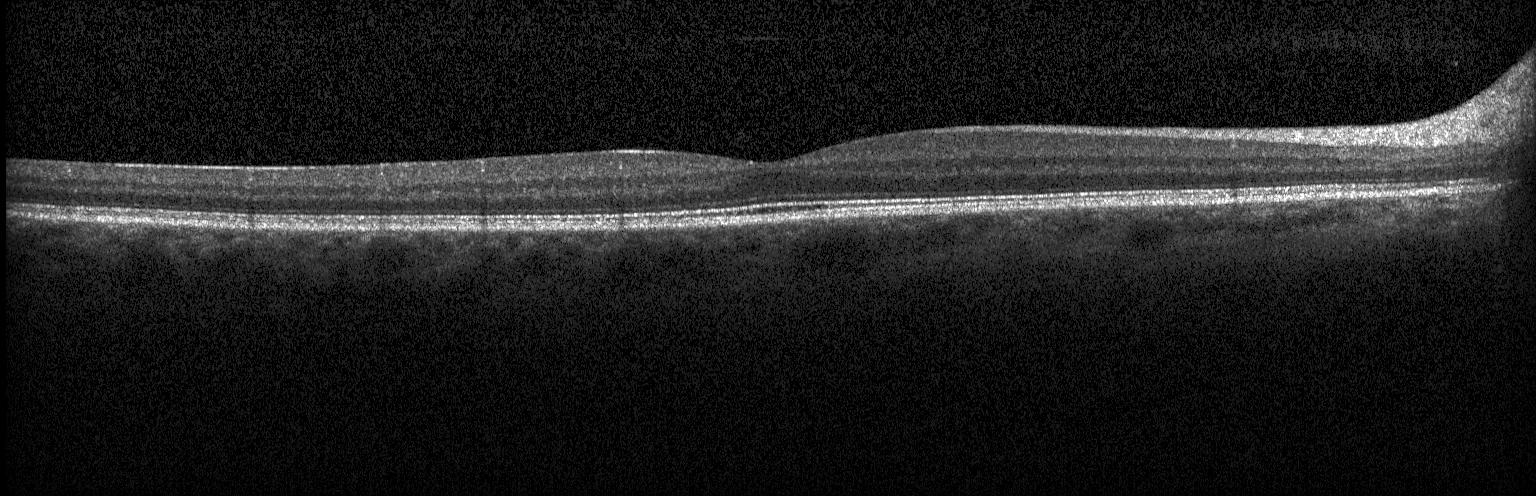
Retinal OCT cross-section, instrument: Heidelberg Spectralis — Diagnosis: no choroidal neovascularization, no diabetic macular edema, and no drusen.